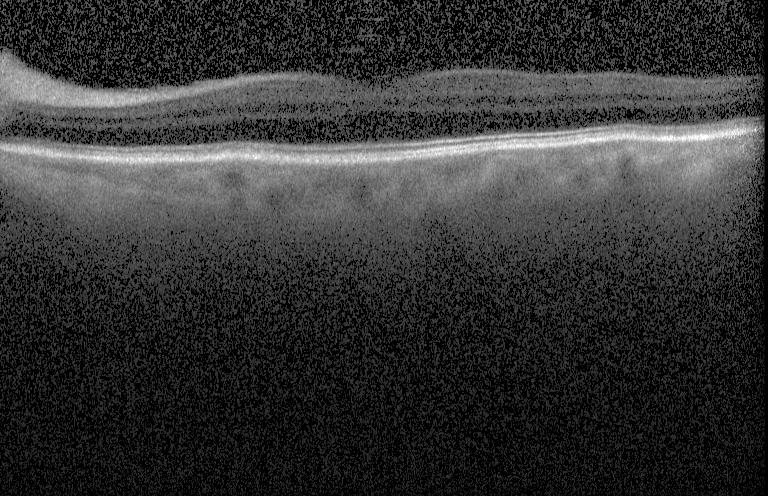 Spectral-domain optical coherence tomography · OCT B-scan. Finding: no choroidal neovascularization, no diabetic macular edema, and no drusen.